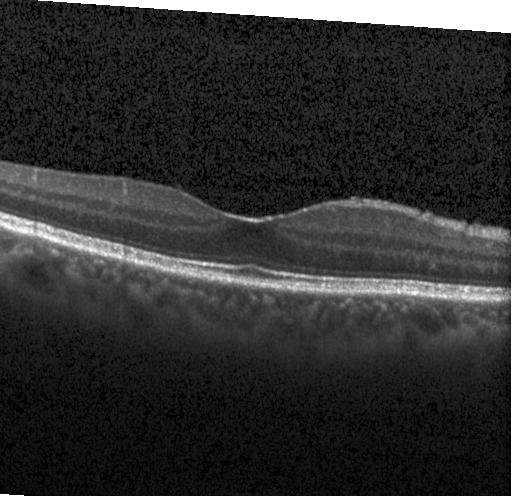 Spectral-domain optical coherence tomography; optical coherence tomography B-scan; instrument: Heidelberg Spectralis; fovea-centered — Finding: no CNV, no DME, and no drusen.